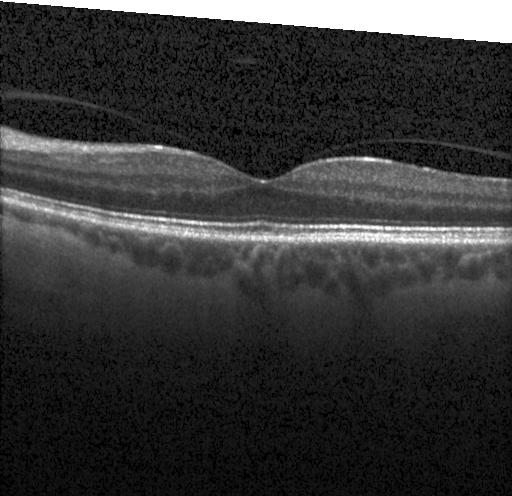 Fovea-centered · spectral-domain OCT · optical coherence tomography B-scan · Heidelberg Spectralis OCT system
OCT finding: no choroidal neovascularization, no diabetic macular edema, and no drusen.